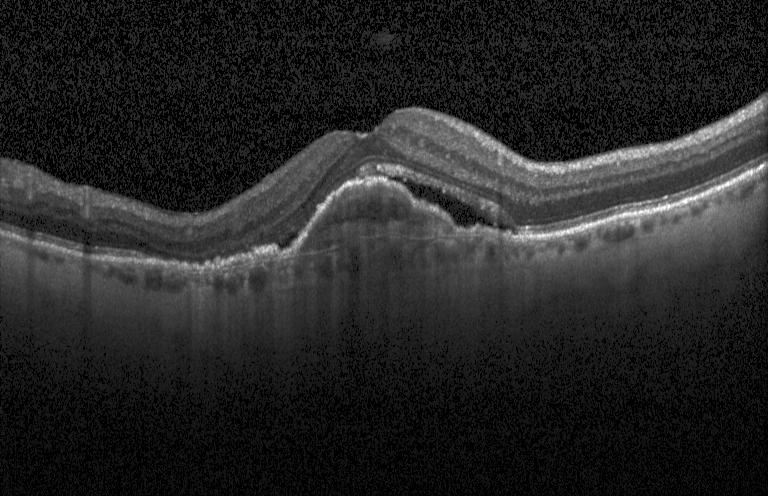

The scan shows CNV.